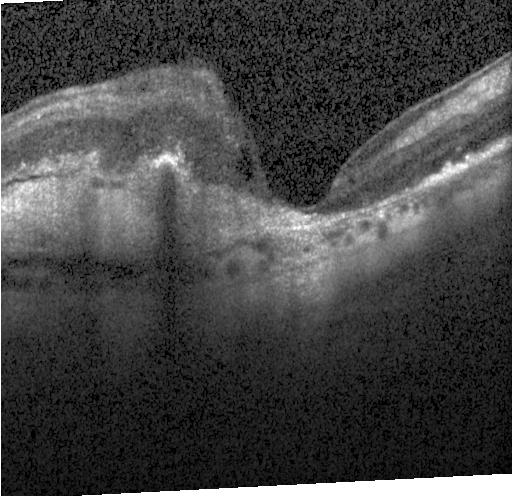

OCT B-scan showing CNV.